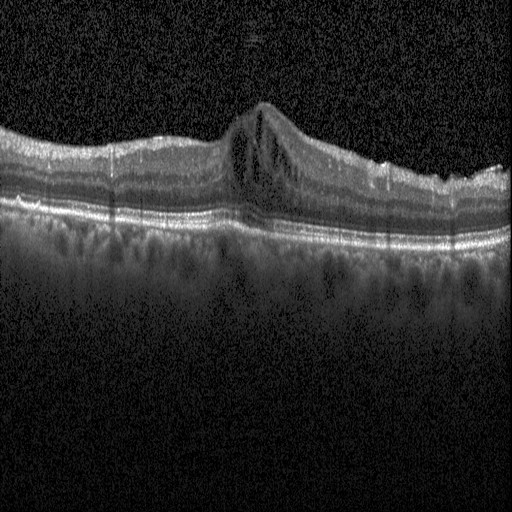

Heidelberg Spectralis OCT system · spectral-domain OCT · OCT line scan · centered on the fovea — Finding: diabetic macular edema (DME).